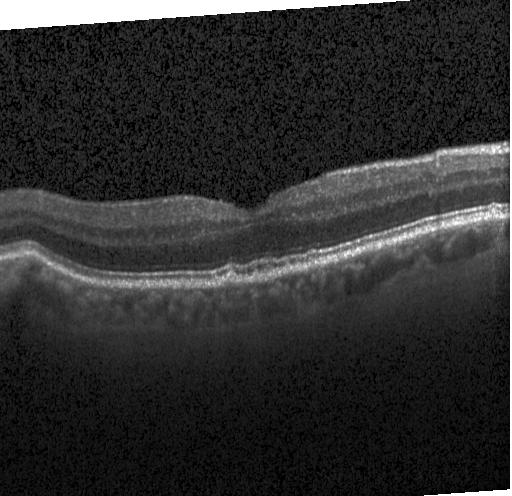

Heidelberg Spectralis OCT system, optical coherence tomography scan, spectral-domain OCT, through the macula. Assessment: sub-RPE drusenoid deposits.